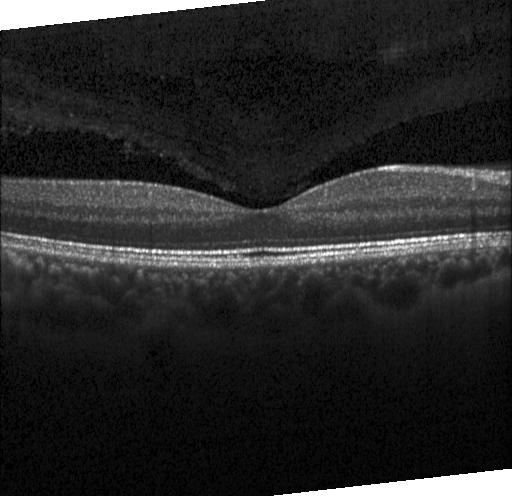 Diagnosis: no choroidal neovascularization, no diabetic macular edema, and no drusen.